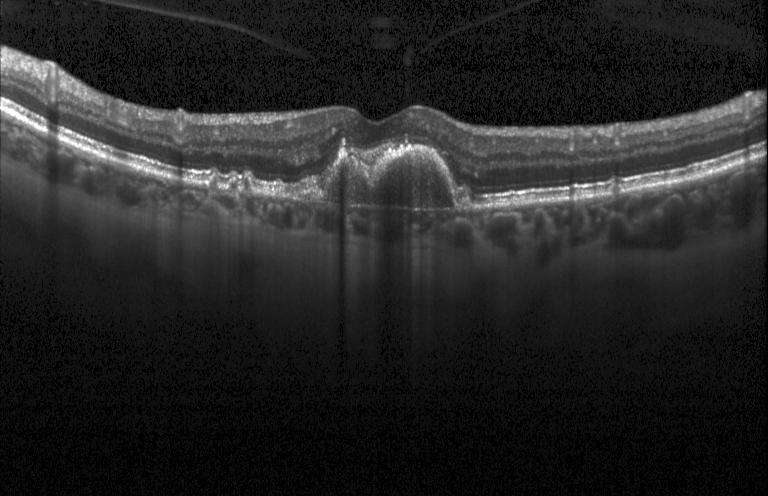

Instrument: Heidelberg Spectralis; centered on the fovea; optical coherence tomography scan
This B-scan demonstrates a choroidal neovascular membrane.